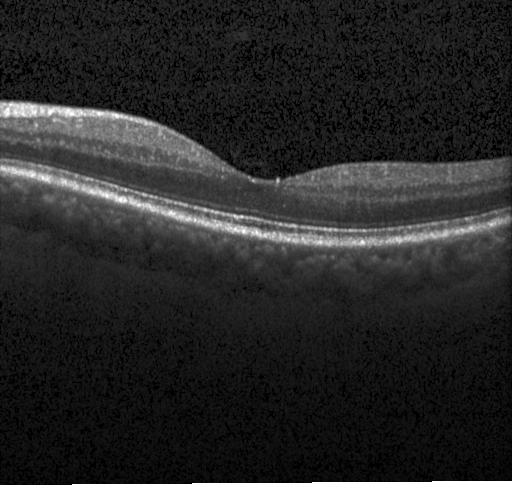
Macular OCT: no choroidal neovascularization, no diabetic macular edema, and no drusen.